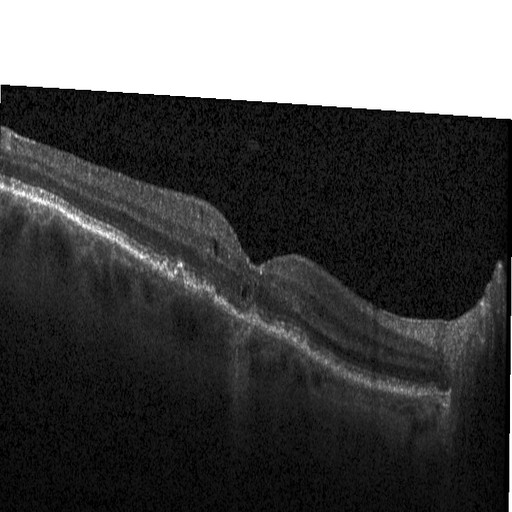
Retinal OCT cross-section.
The scan shows diabetic macular edema (DME).